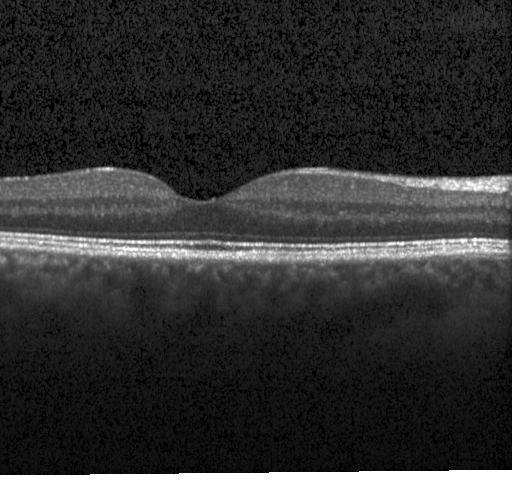 Heidelberg Spectralis OCT system. Spectral-domain optical coherence tomography. Retinal OCT cross-section
Impression: no evidence of CNV, DME, or drusen.